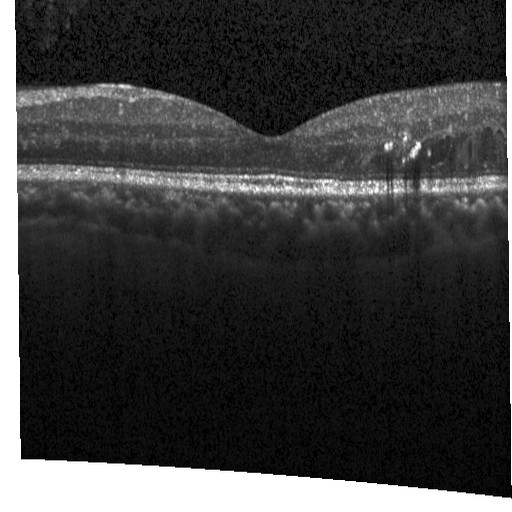 OCT line scan
This B-scan demonstrates diabetic macular edema.